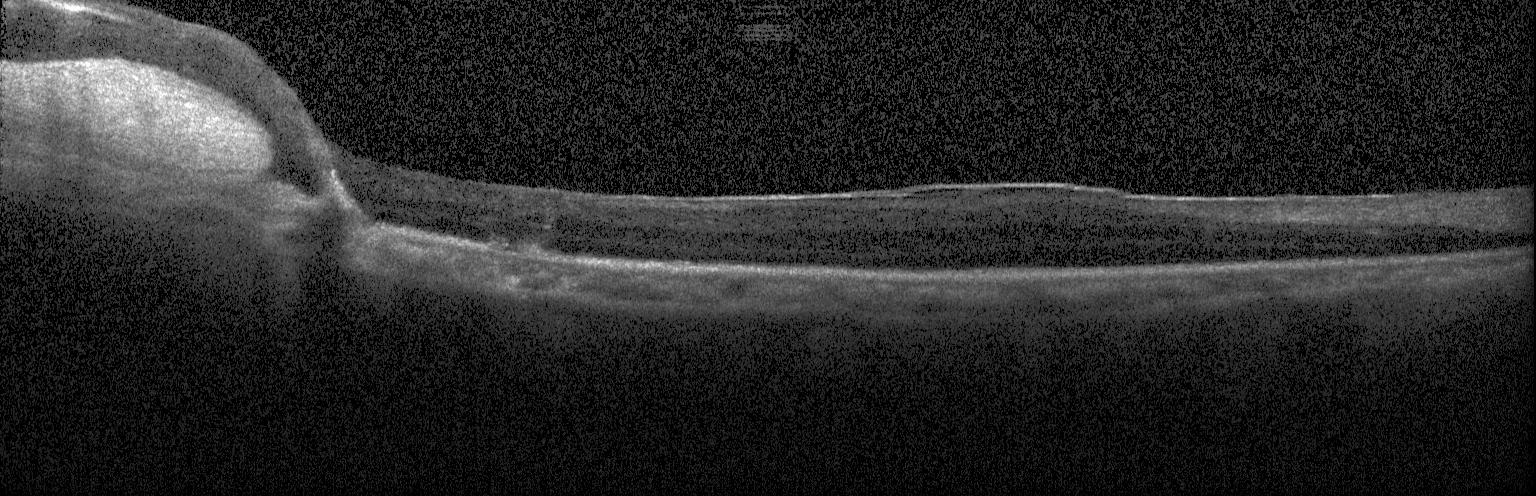
Choroidal neovascularization.